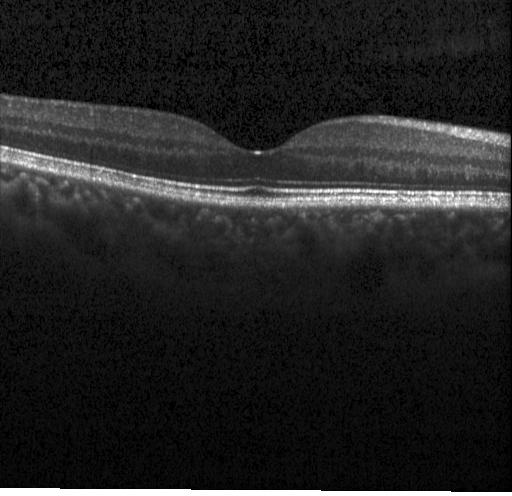
Optical coherence tomography scan · through the macula · acquired on a Heidelberg Spectralis — Diagnosis: neither choroidal neovascularization, diabetic macular edema, nor drusen.